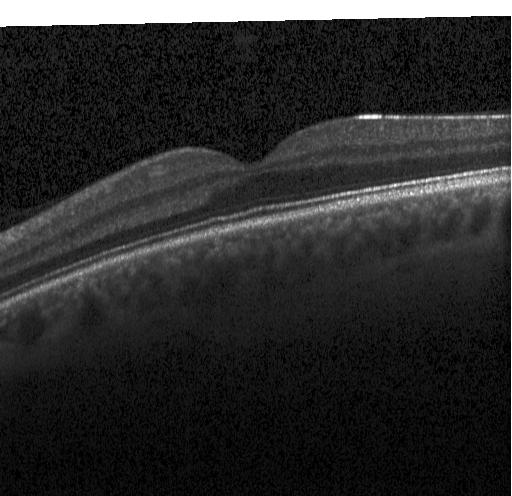 SD-OCT; acquired on a Heidelberg Spectralis; fovea-centered; optical coherence tomography scan.
OCT finding: neither CNV, DME, nor drusen.